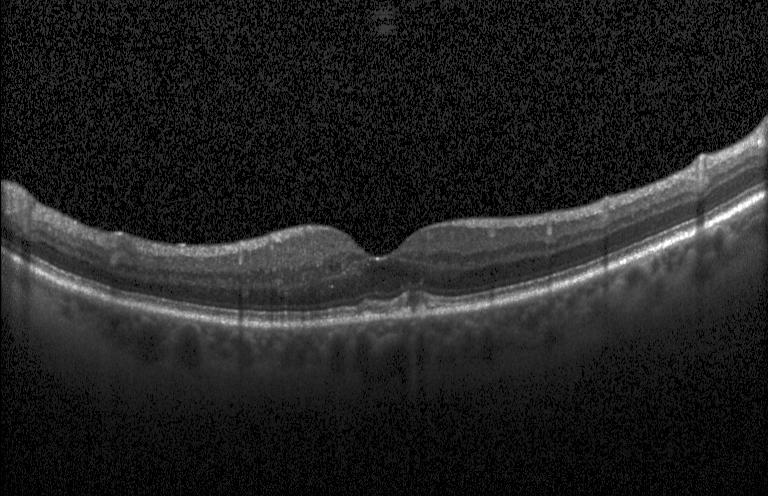
Instrument: Heidelberg Spectralis · optical coherence tomography scan · horizontal scan through the fovea — Assessment: multiple drusen.